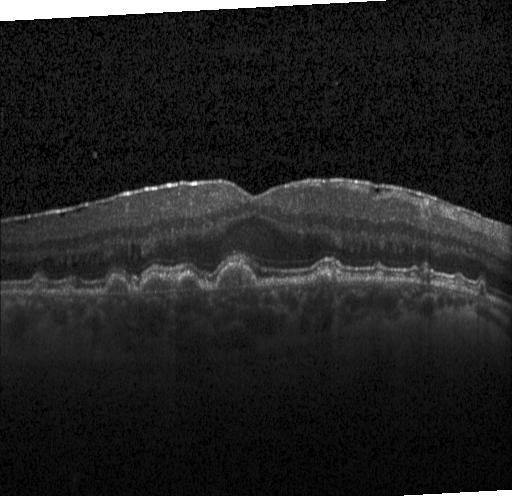 Assessment: sub-RPE drusenoid deposits.